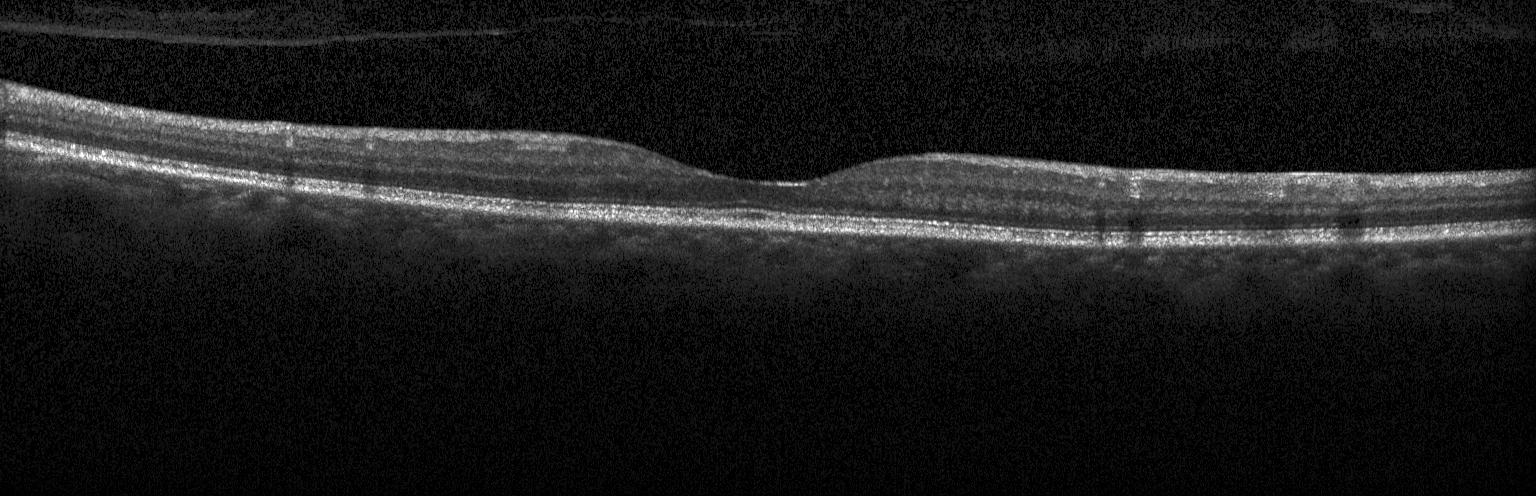 OCT line scan
No CNV, no DME, and no drusen.